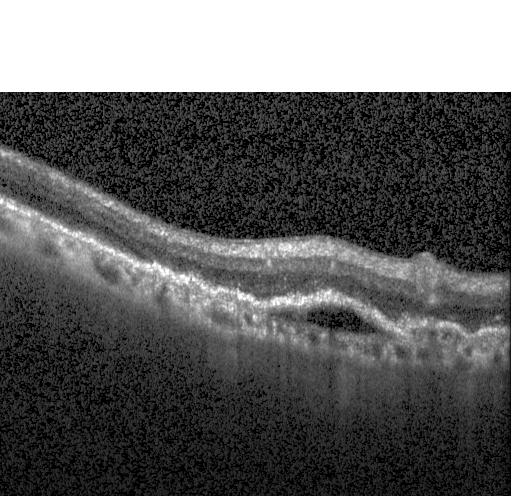

Heidelberg Spectralis · OCT line scan · SD-OCT · horizontal scan through the fovea
This B-scan demonstrates CNV.